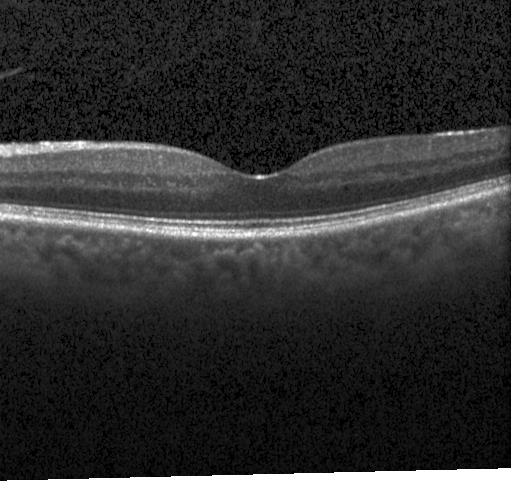 Finding: no evidence of CNV, DME, or drusen.